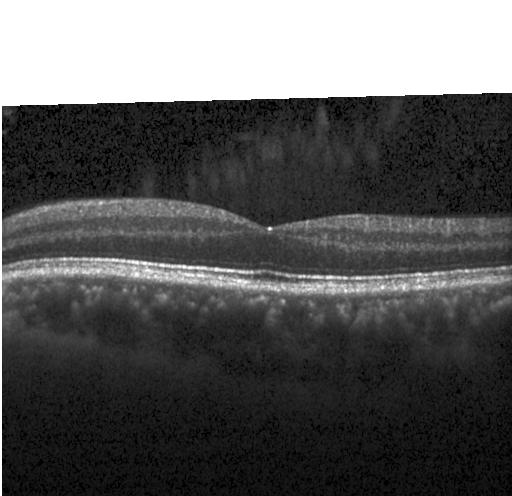 Optical coherence tomography B-scan. Instrument: Heidelberg Spectralis. Diagnosis: no choroidal neovascularization, no diabetic macular edema, and no drusen.